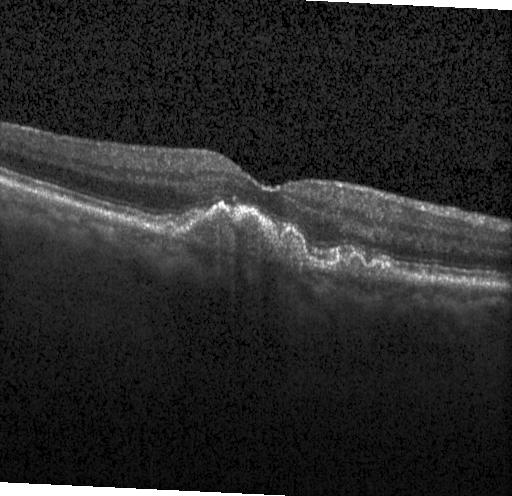 Macular OCT: a choroidal neovascular membrane.